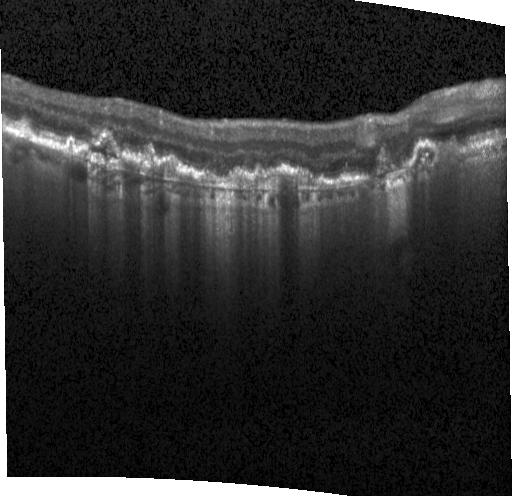

Diagnosis: CNV.